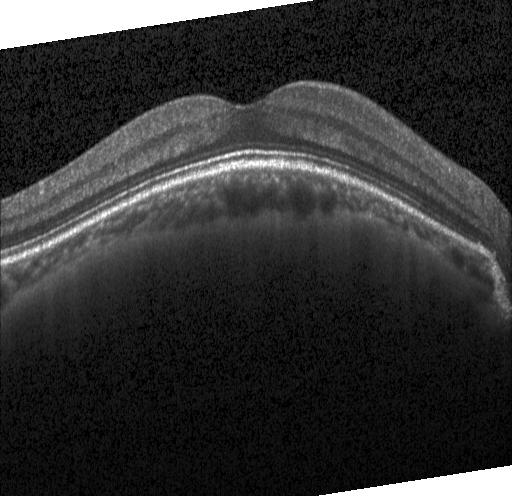
Fovea-centered. SD-OCT. OCT B-scan. Impression: neither choroidal neovascularization, diabetic macular edema, nor drusen.